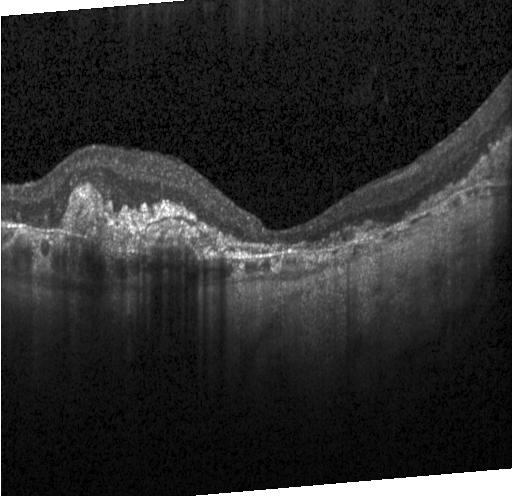

Retinal OCT B-scan, spectral-domain optical coherence tomography, acquired on a Heidelberg Spectralis.
Finding: a choroidal neovascular membrane.